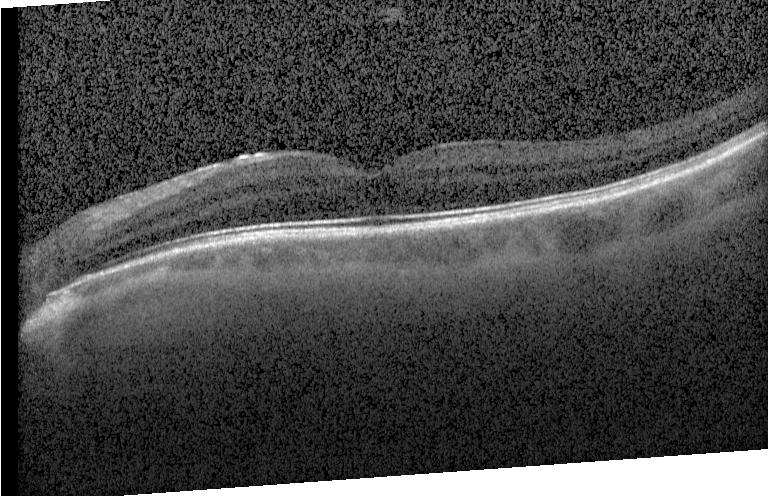
Macular scan. OCT B-scan. Spectral-domain OCT — This B-scan demonstrates no evidence of choroidal neovascularization, diabetic macular edema, or drusen.